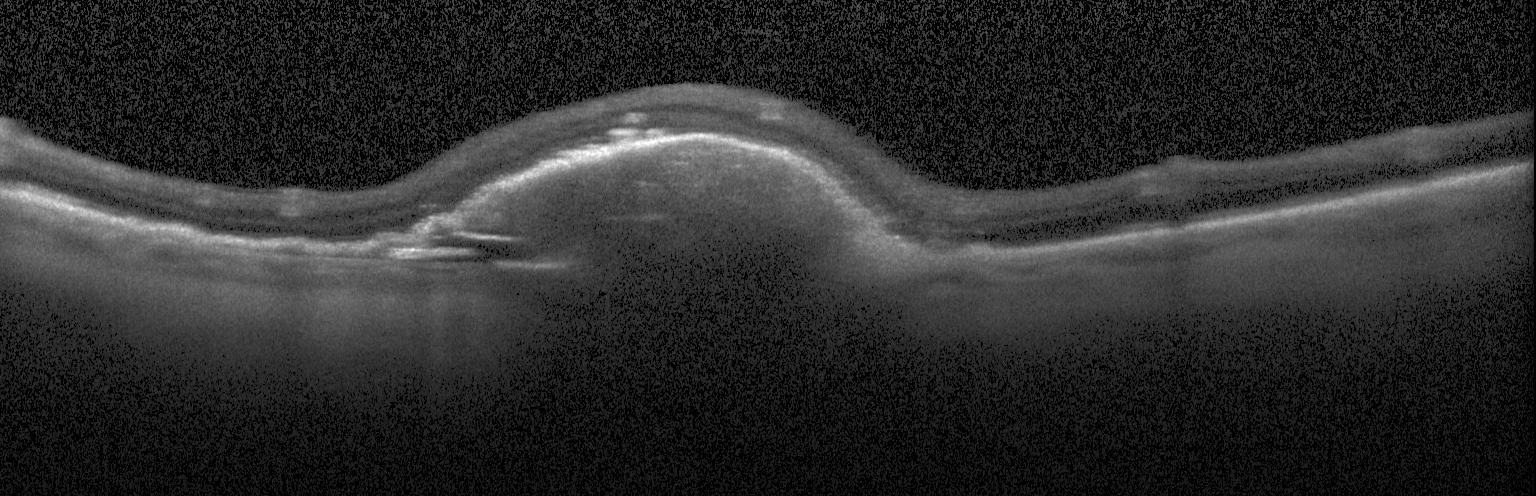
Impression: a choroidal neovascular membrane.